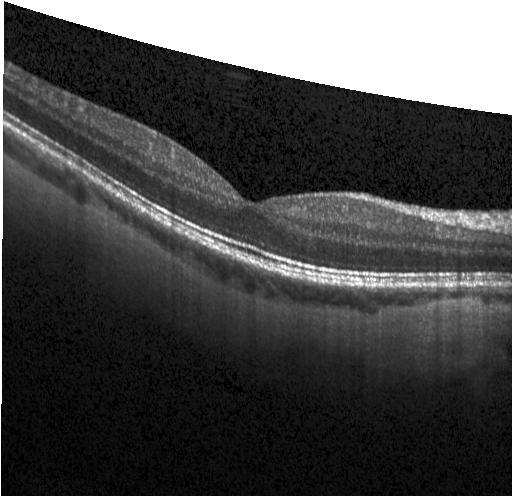
OCT line scan.
Impression: no CNV, no DME, and no drusen.